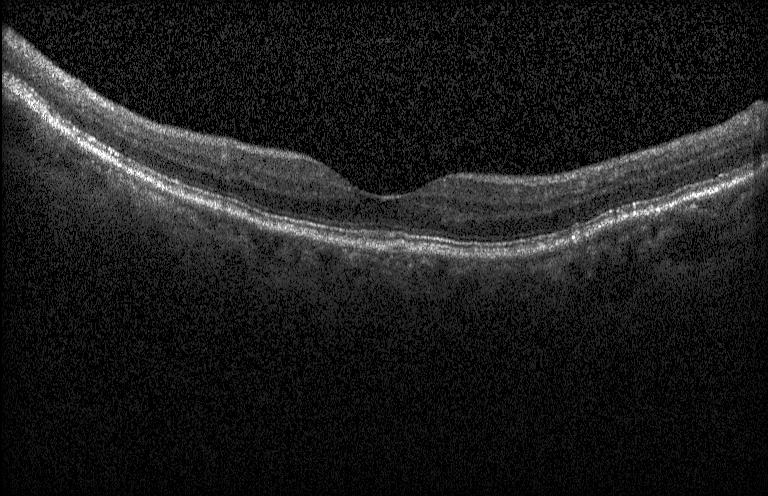 Impression: no choroidal neovascularization, diabetic macular edema, or drusen.